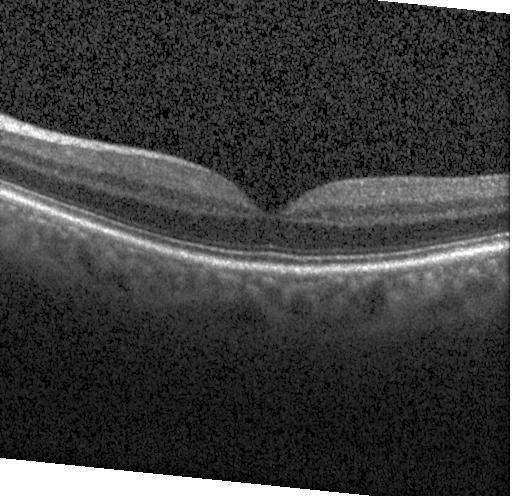 Finding: neither choroidal neovascularization, diabetic macular edema, nor drusen.